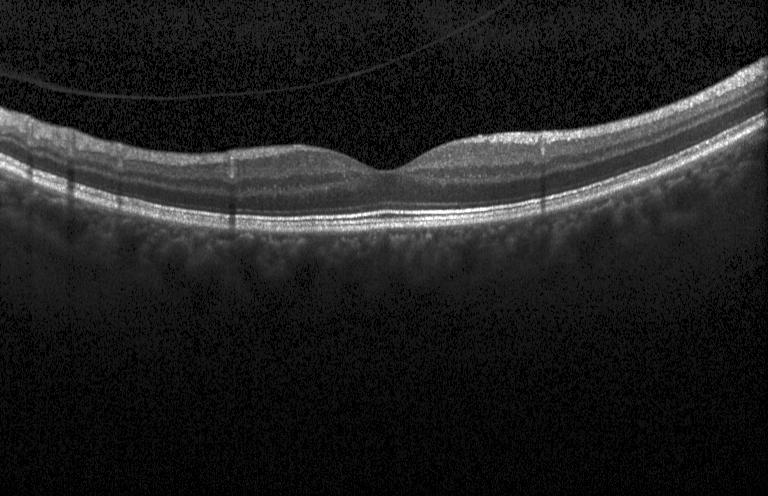 SD-OCT; retinal OCT B-scan; Heidelberg Spectralis
Assessment: no choroidal neovascularization, no diabetic macular edema, and no drusen.